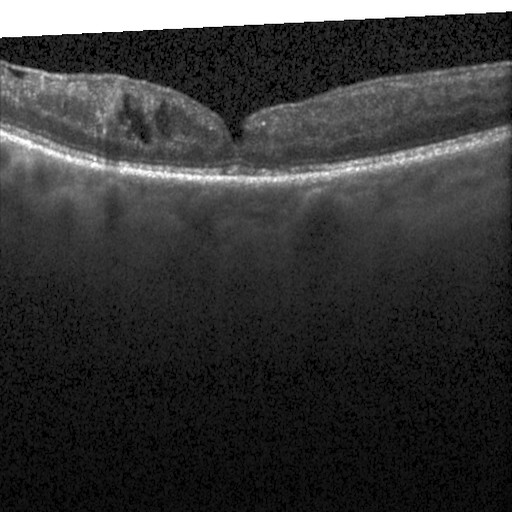 Spectral-domain optical coherence tomography; through the macula; retinal OCT B-scan — Finding: diabetic macular edema (DME).